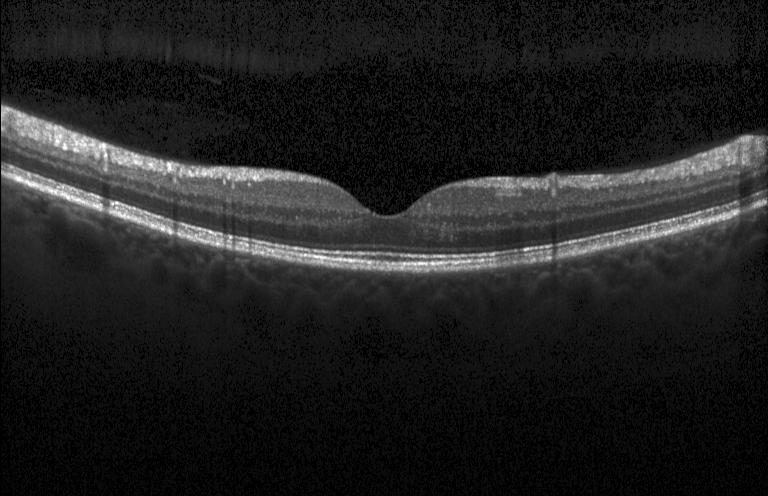 Spectral-domain optical coherence tomography; retinal OCT cross-section; instrument: Heidelberg Spectralis
Finding: no evidence of choroidal neovascularization, diabetic macular edema, or drusen.